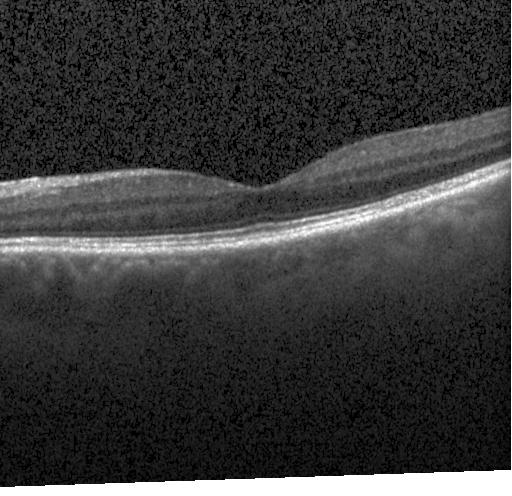 Finding: no evidence of choroidal neovascularization, diabetic macular edema, or drusen.